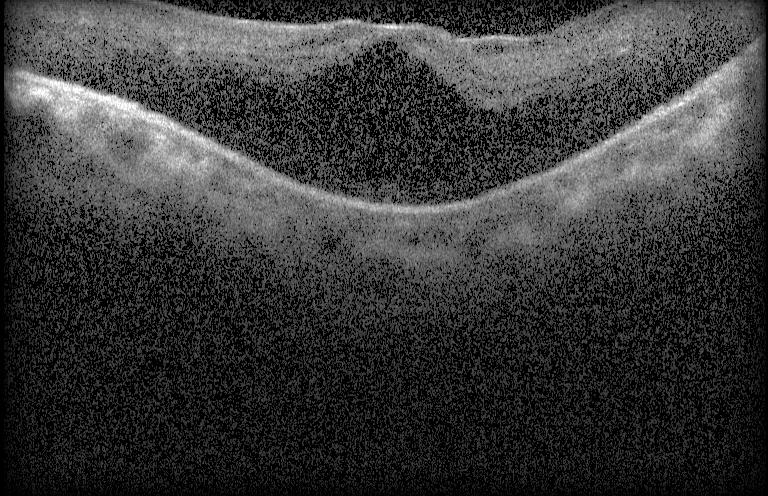 Retinal OCT cross-section. Impression: diabetic macular edema.